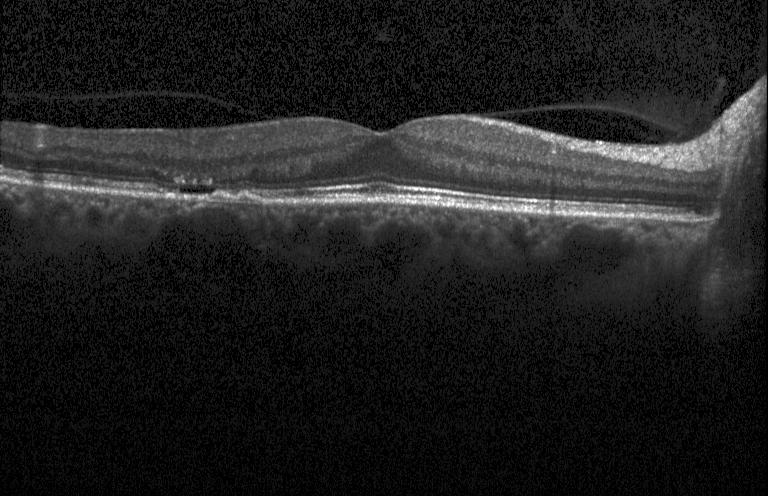

Heidelberg Spectralis; OCT B-scan; spectral-domain optical coherence tomography
Diagnosis: a choroidal neovascular membrane.